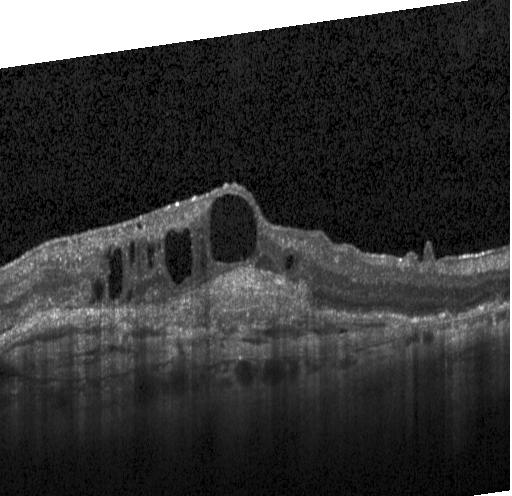
Optical coherence tomography scan. Spectral-domain optical coherence tomography.
Finding: a choroidal neovascular membrane.